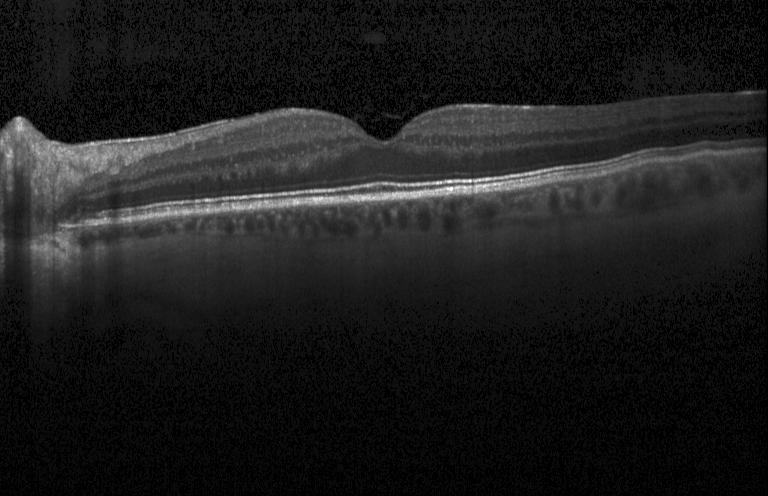 Through the macula. Spectral-domain OCT. OCT B-scan
Diagnosis: no choroidal neovascularization, diabetic macular edema, or drusen.